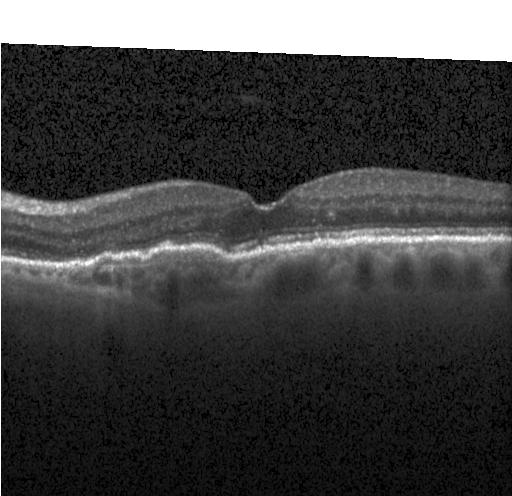

Choroidal neovascularization (CNV).